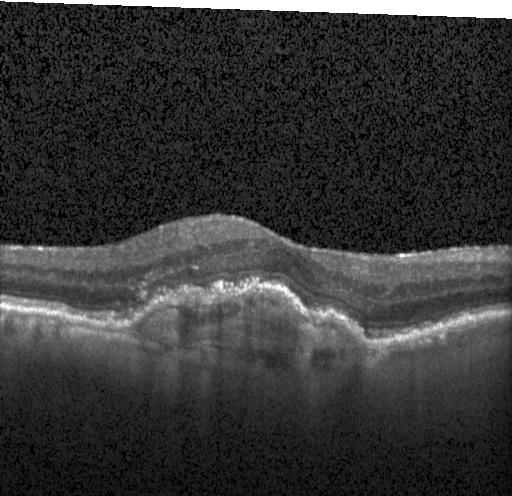
Diagnosis: choroidal neovascularization.